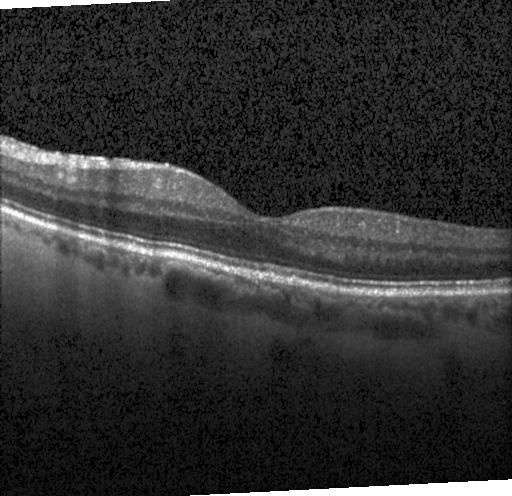 OCT B-scan.
Finding: no choroidal neovascularization, diabetic macular edema, or drusen.